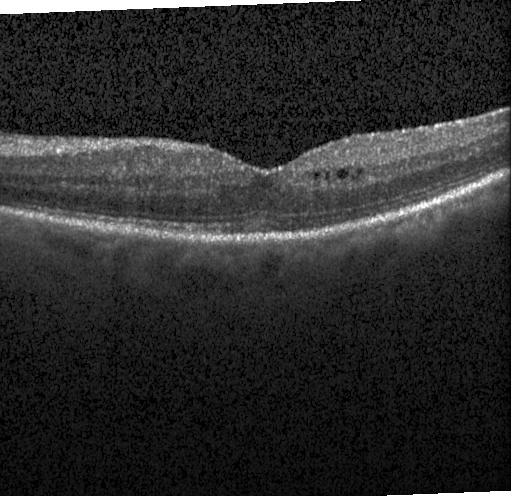
Retinal OCT cross-section showing DME.